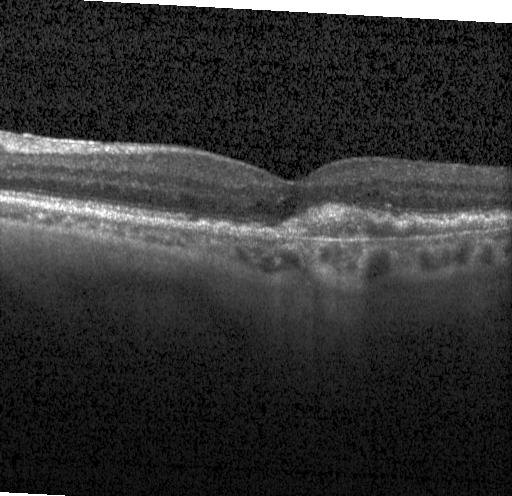 OCT B-scan
Impression: a choroidal neovascular membrane.